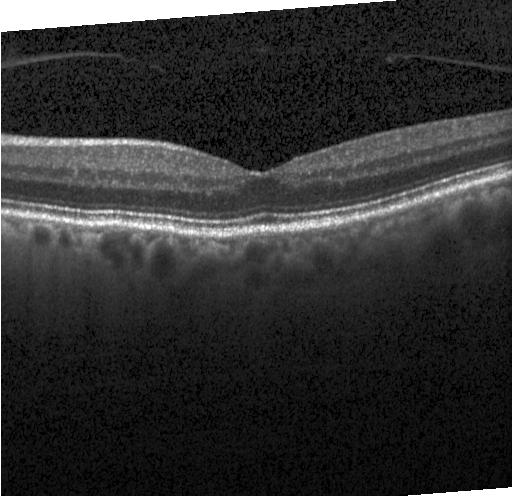 Horizontal scan through the fovea. Retinal OCT cross-section — This B-scan demonstrates neither choroidal neovascularization, diabetic macular edema, nor drusen.